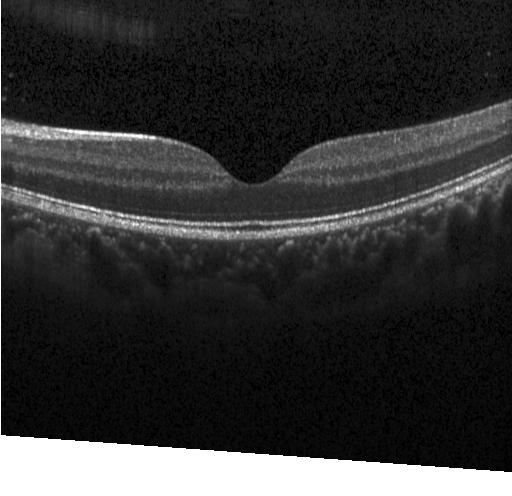 OCT B-scan showing no evidence of choroidal neovascularization, diabetic macular edema, or drusen.